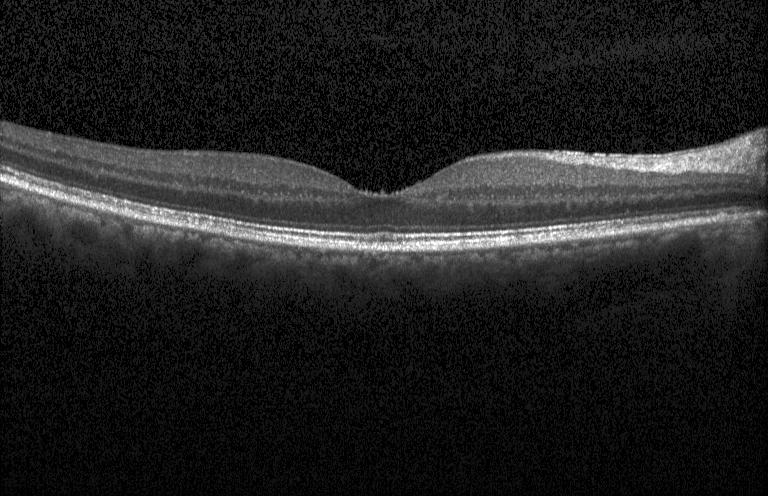 Retinal OCT cross-section showing neither choroidal neovascularization, diabetic macular edema, nor drusen.